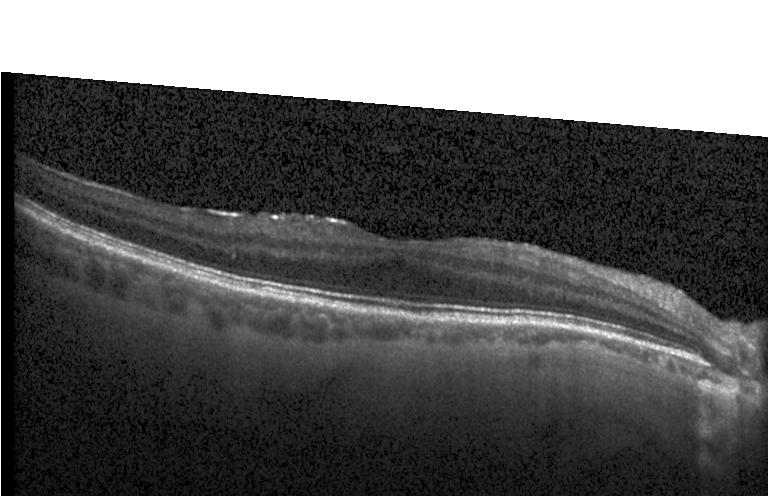 Spectral-domain OCT; horizontal scan through the fovea; retinal OCT B-scan
Finding: no CNV, no DME, and no drusen.